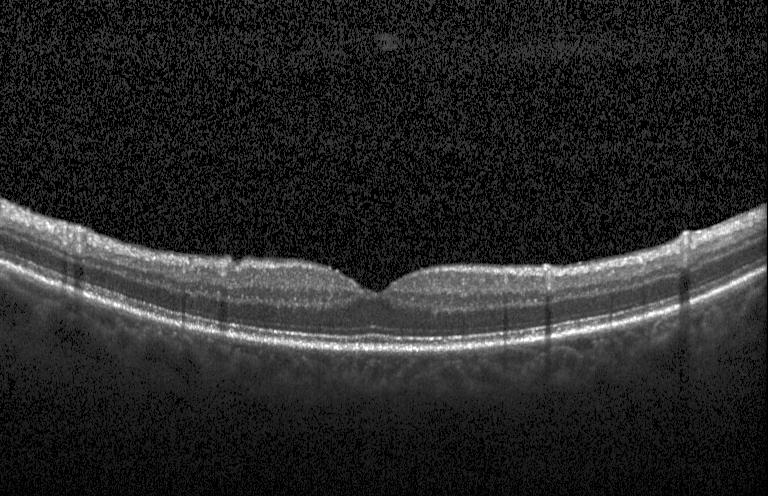 OCT finding: no choroidal neovascularization, diabetic macular edema, or drusen.